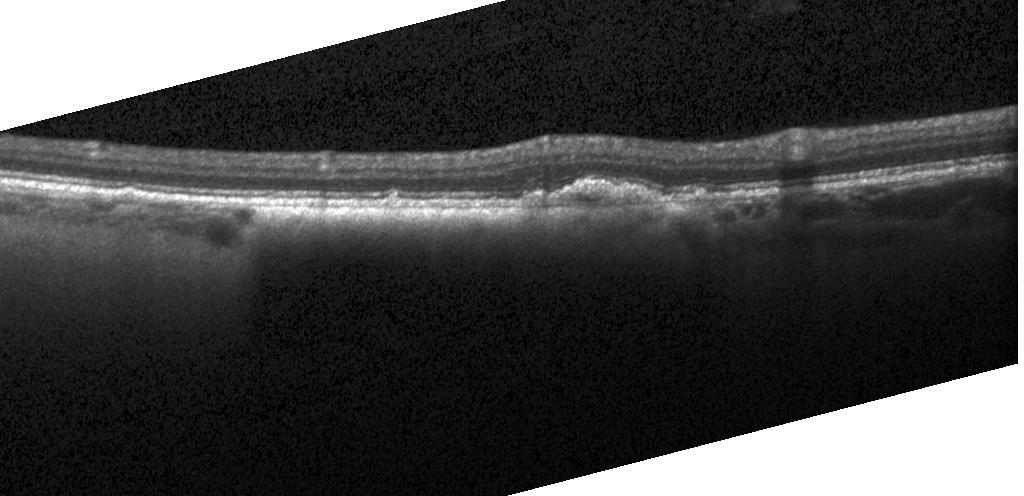

Retinal OCT cross-section showing choroidal neovascularization.